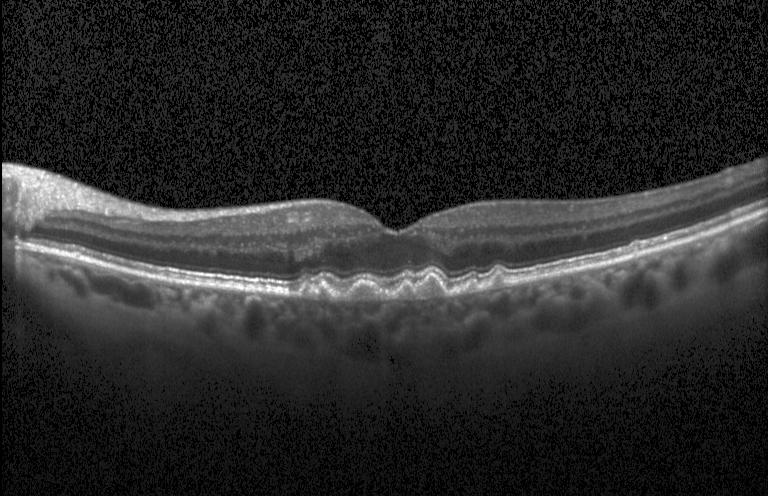

OCT line scan. Macular OCT: drusen.